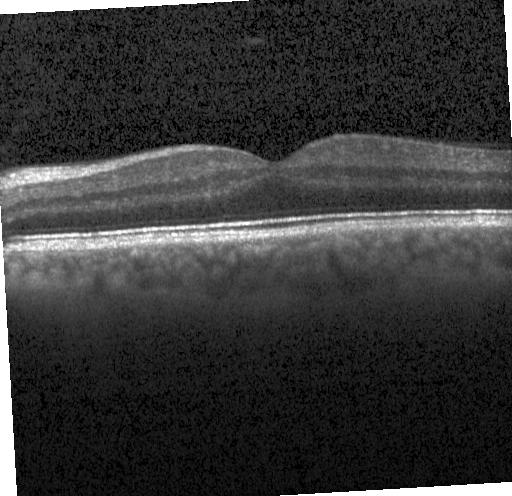
Spectral-domain OCT · fovea-centered · optical coherence tomography scan · acquired on a Heidelberg Spectralis — Assessment: neither choroidal neovascularization, diabetic macular edema, nor drusen.